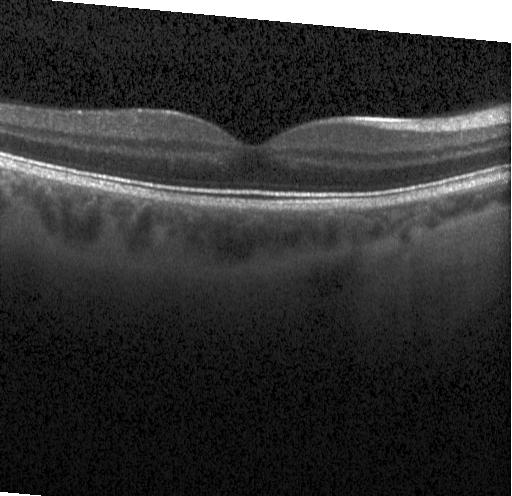 Optical coherence tomography B-scan
Finding: no choroidal neovascularization, no diabetic macular edema, and no drusen.